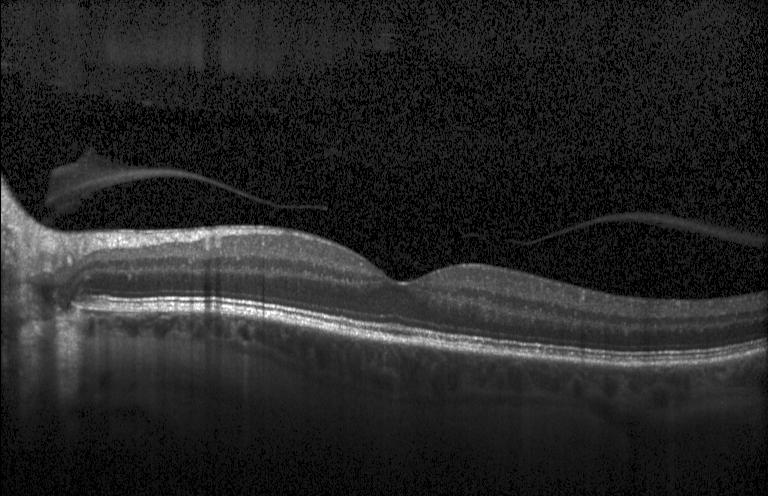 Impression: neither CNV, DME, nor drusen.